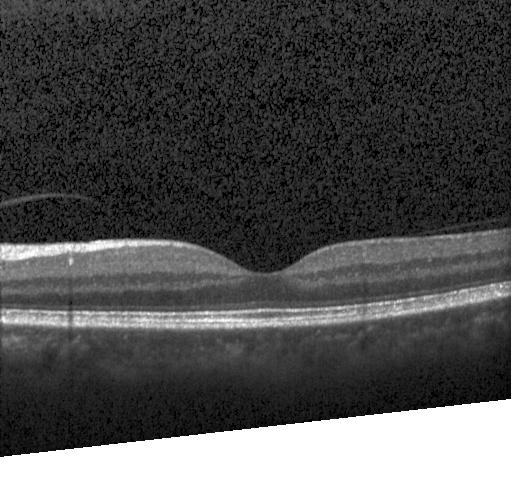

Retinal OCT cross-section showing no evidence of choroidal neovascularization, diabetic macular edema, or drusen.